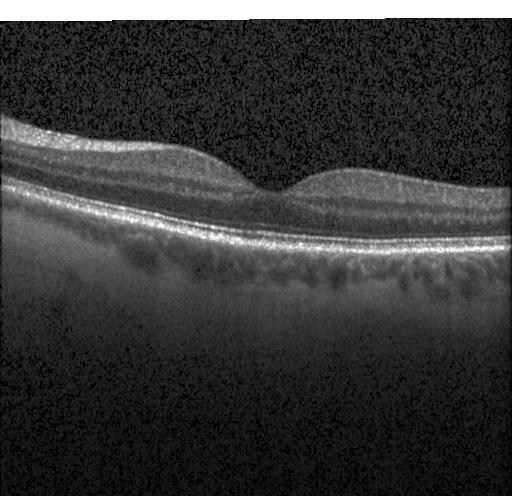
Optical coherence tomography scan · fovea-centered · SD-OCT — Impression: neither choroidal neovascularization, diabetic macular edema, nor drusen.